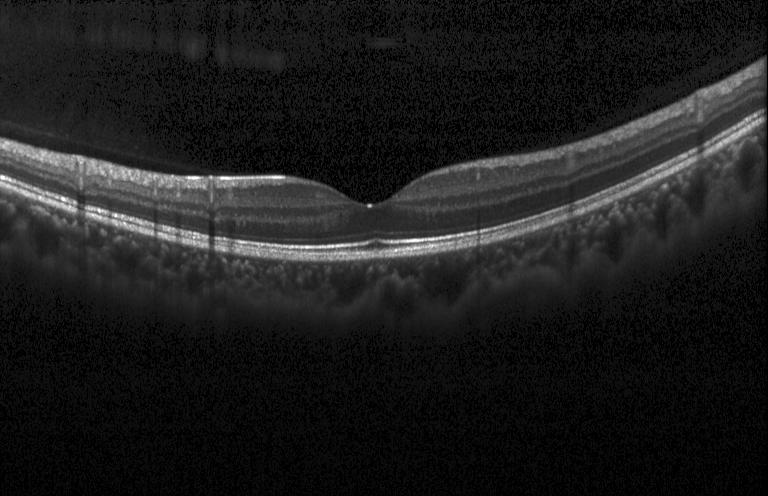
OCT finding: no choroidal neovascularization, no diabetic macular edema, and no drusen.